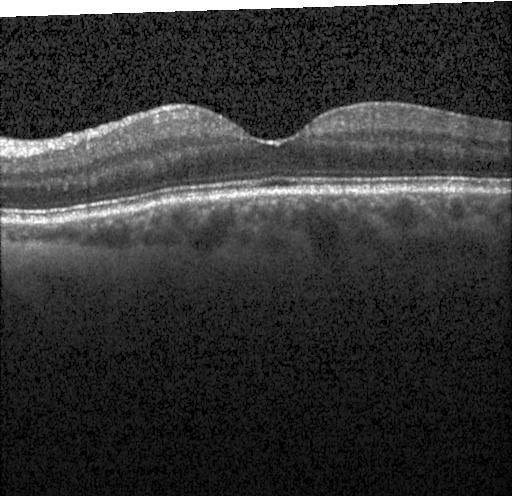

The scan shows no evidence of choroidal neovascularization, diabetic macular edema, or drusen.